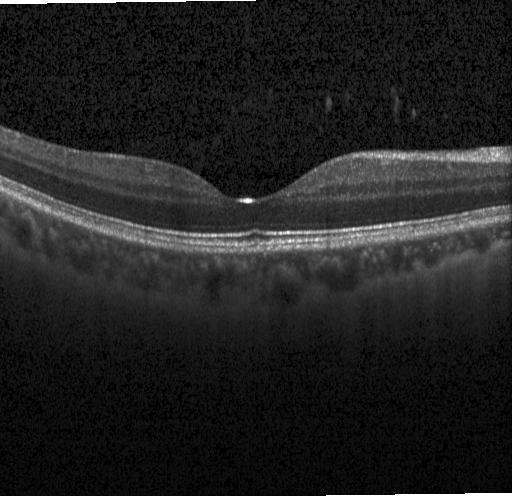

The scan shows no evidence of choroidal neovascularization, diabetic macular edema, or drusen.